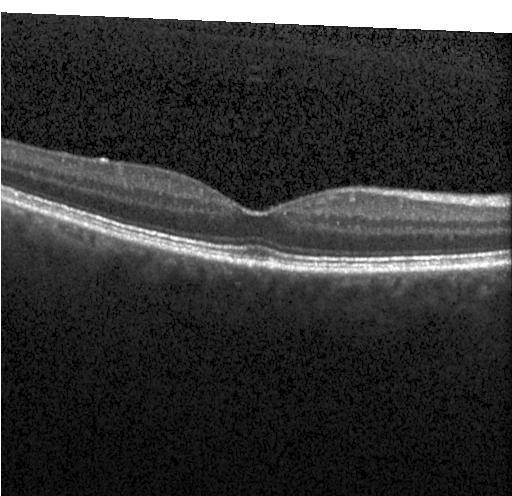 OCT finding: no evidence of CNV, DME, or drusen.